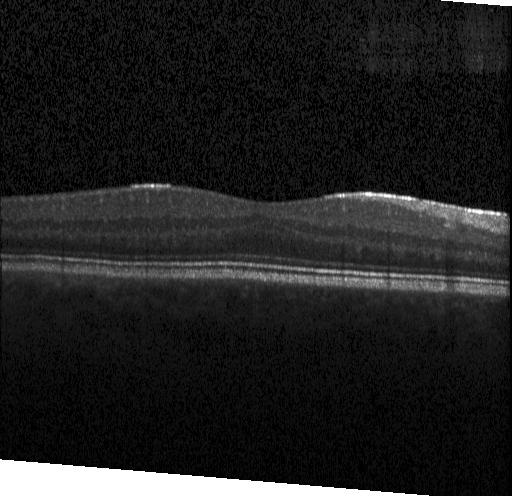
OCT B-scan. OCT finding: no CNV, DME, or drusen.